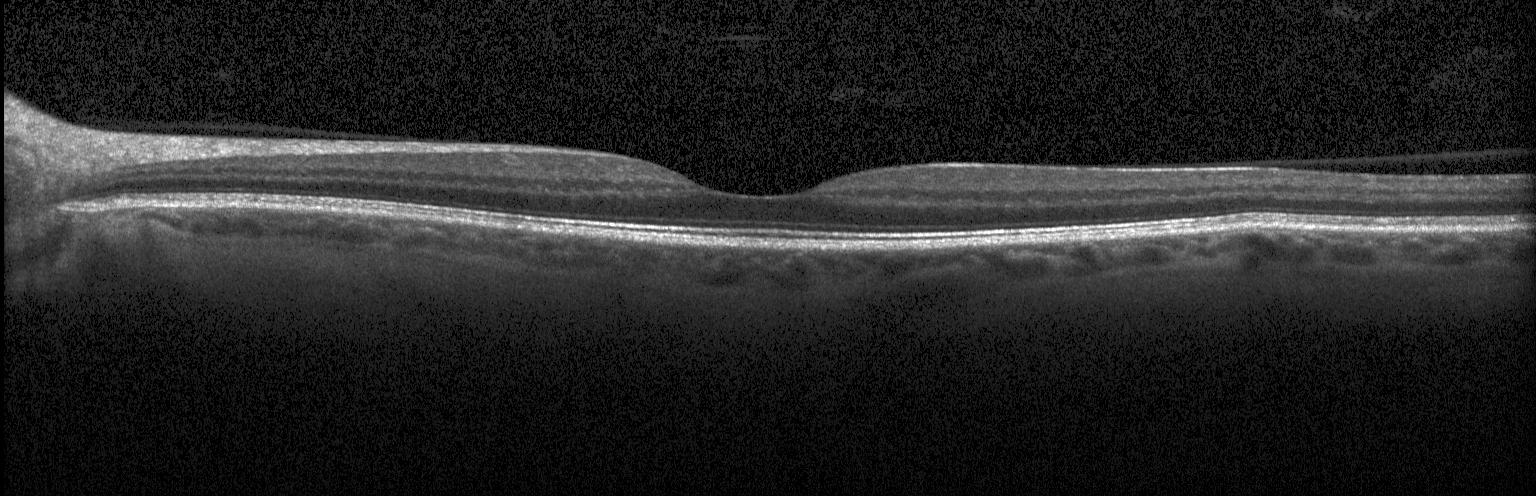
Retinal OCT cross-section — Finding: neither choroidal neovascularization, diabetic macular edema, nor drusen.